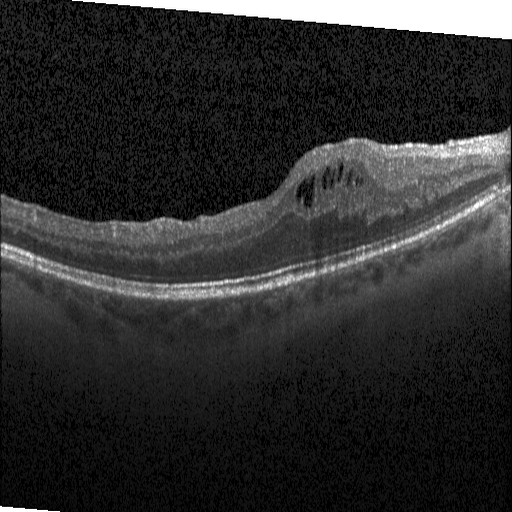

OCT scan showing diabetic macular edema (DME).